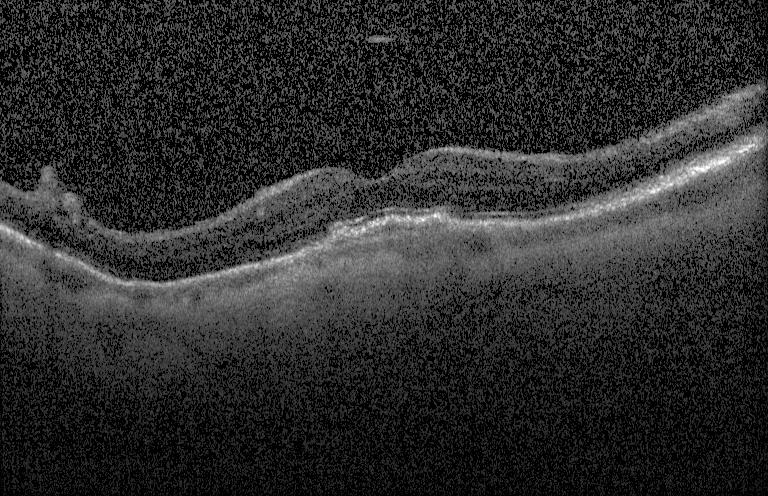
Heidelberg Spectralis OCT system; spectral-domain optical coherence tomography; OCT B-scan
A choroidal neovascular membrane.